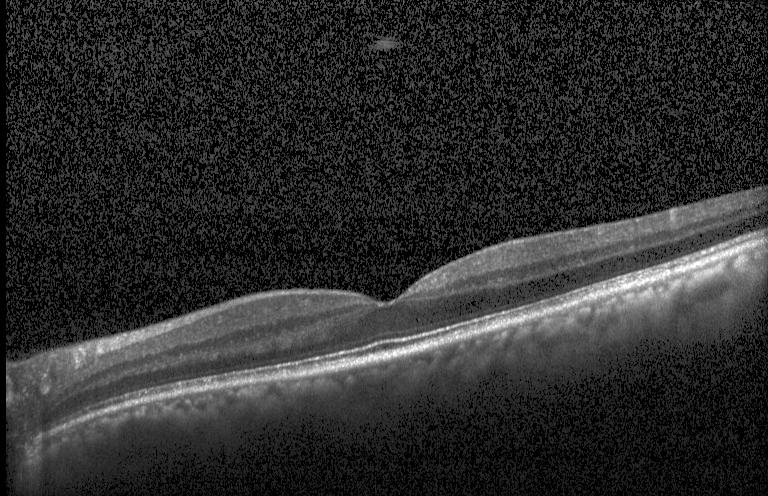

Spectral-domain optical coherence tomography. Optical coherence tomography B-scan.
Assessment: no CNV, no DME, and no drusen.